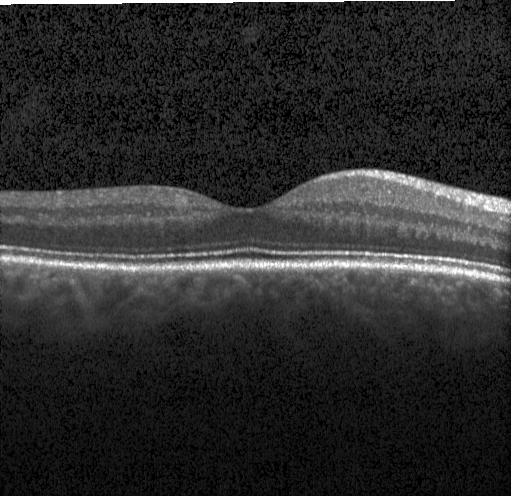 OCT B-scan. Acquired on a Heidelberg Spectralis. Macular scan. SD-OCT. Finding: no choroidal neovascularization, no diabetic macular edema, and no drusen.